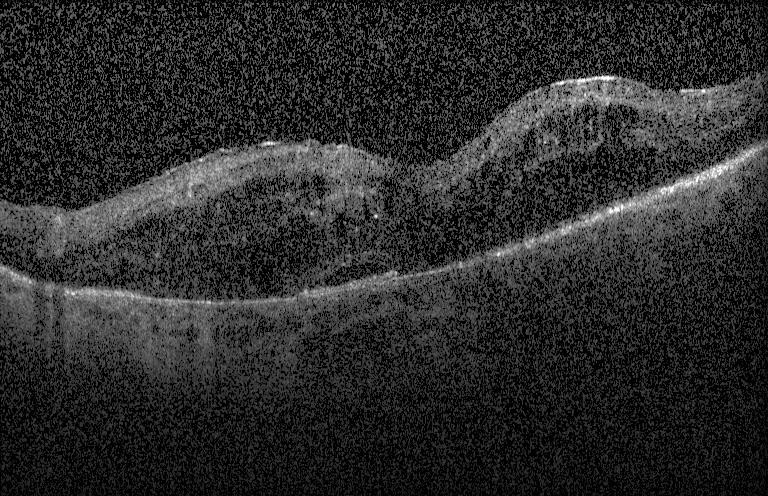

Heidelberg Spectralis OCT system, SD-OCT, retinal OCT B-scan.
Diagnosis: choroidal neovascularization.